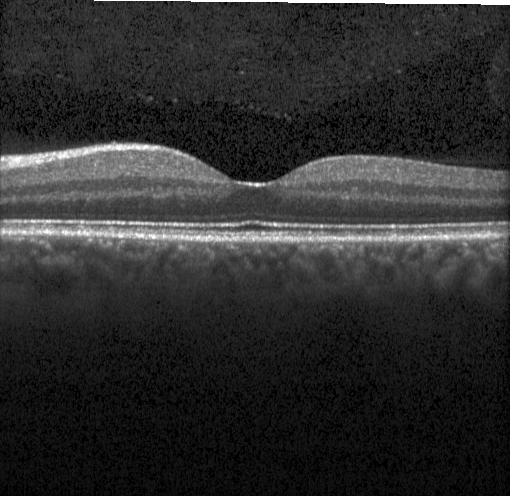 Spectral-domain OCT B-scan: neither choroidal neovascularization, diabetic macular edema, nor drusen.